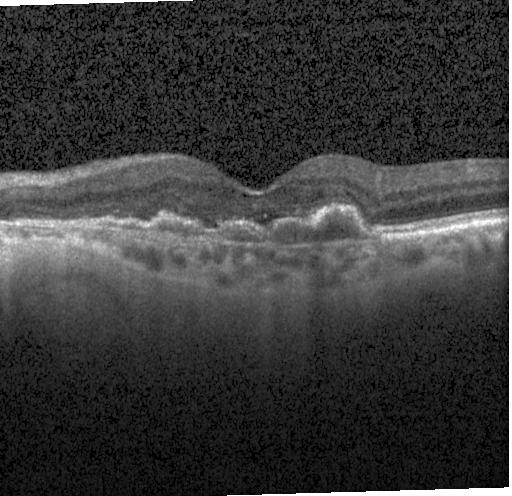
Macular OCT demonstrating a choroidal neovascular membrane.